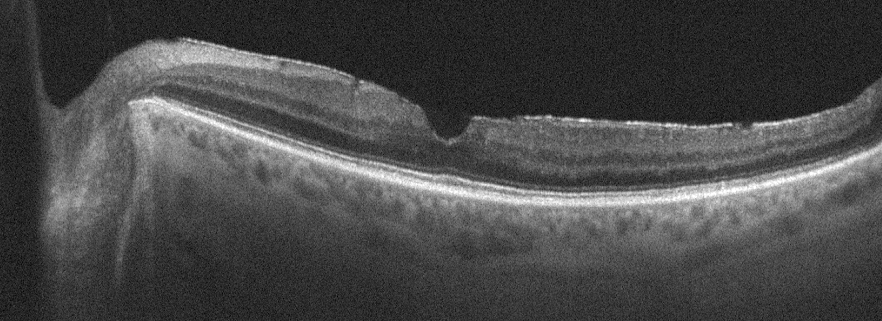
This B-scan demonstrates epiretinal membrane (ERM).